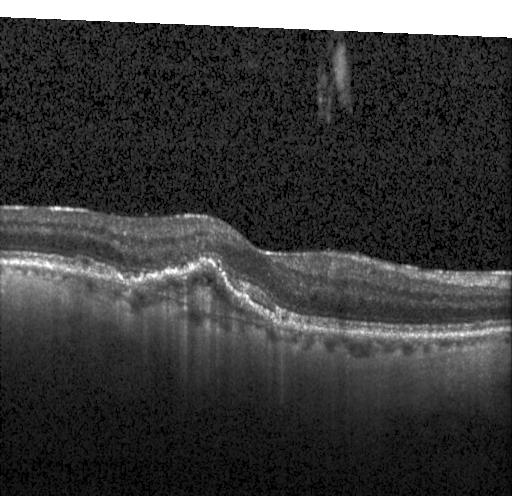
SD-OCT; optical coherence tomography B-scan
This B-scan demonstrates choroidal neovascularization.